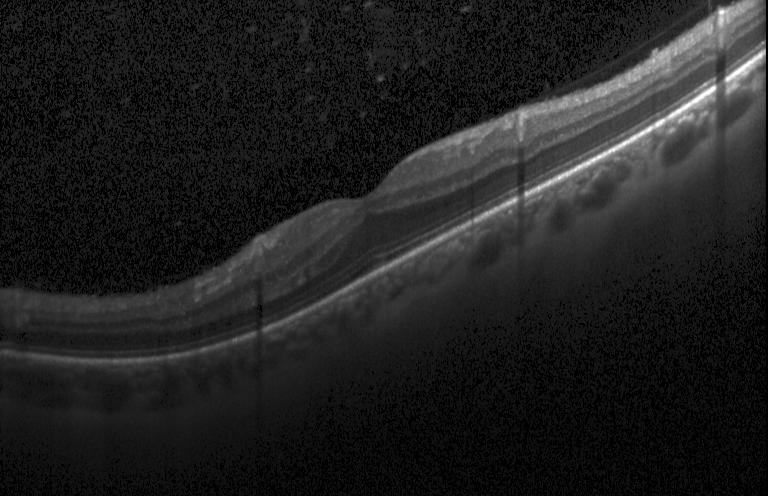

Instrument: Heidelberg Spectralis, retinal OCT cross-section, SD-OCT — No CNV, DME, or drusen.